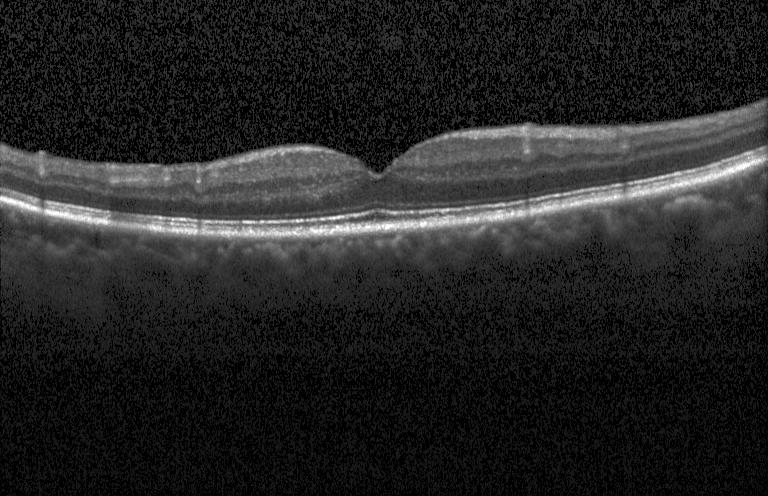 Diagnosis: no CNV, DME, or drusen.